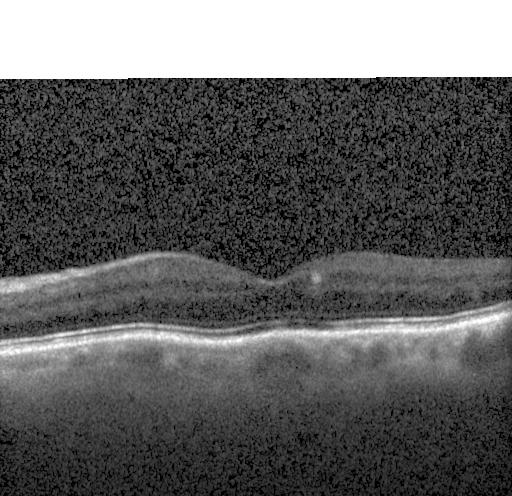
Retinal OCT cross-section; spectral-domain OCT — Diagnosis: no choroidal neovascularization, diabetic macular edema, or drusen.